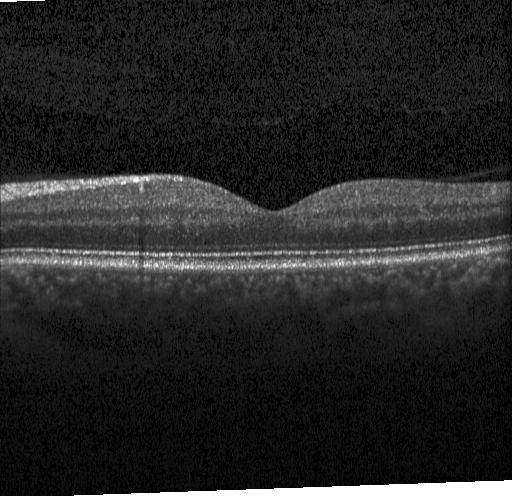

Macular OCT demonstrating no evidence of CNV, DME, or drusen.